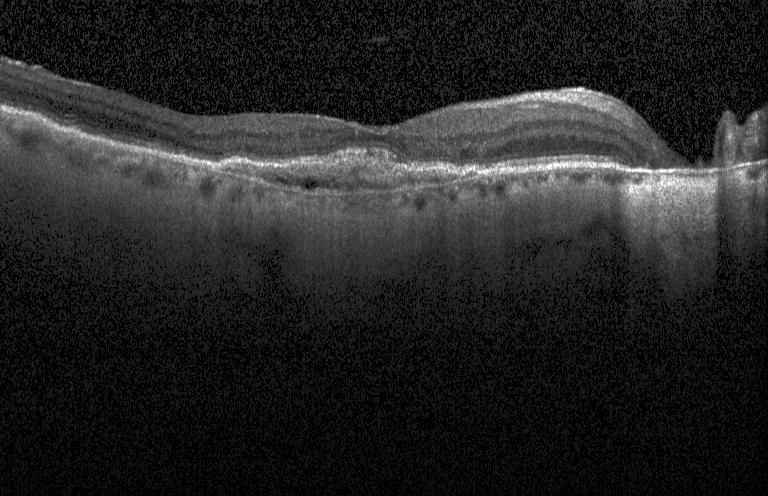 SD-OCT · instrument: Heidelberg Spectralis · OCT line scan · through the macula — A choroidal neovascular membrane.